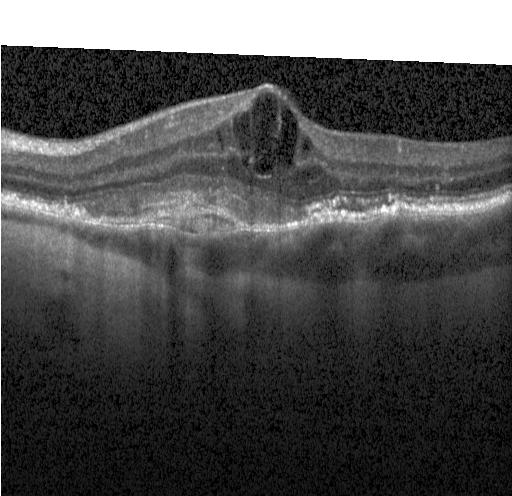

Retinal OCT B-scan, horizontal scan through the fovea, spectral-domain optical coherence tomography. Impression: choroidal neovascularization (CNV).